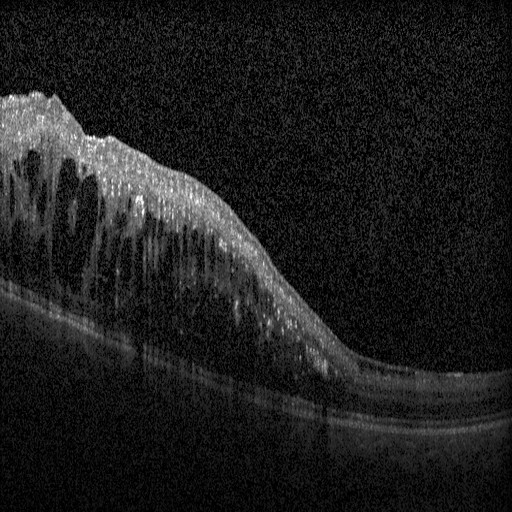 Diabetic macular edema.